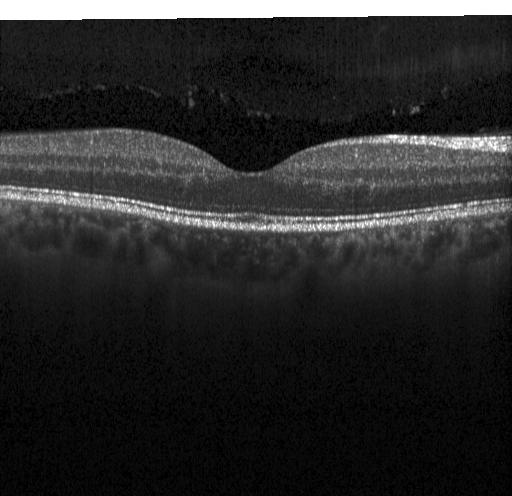
This B-scan demonstrates no choroidal neovascularization, no diabetic macular edema, and no drusen.